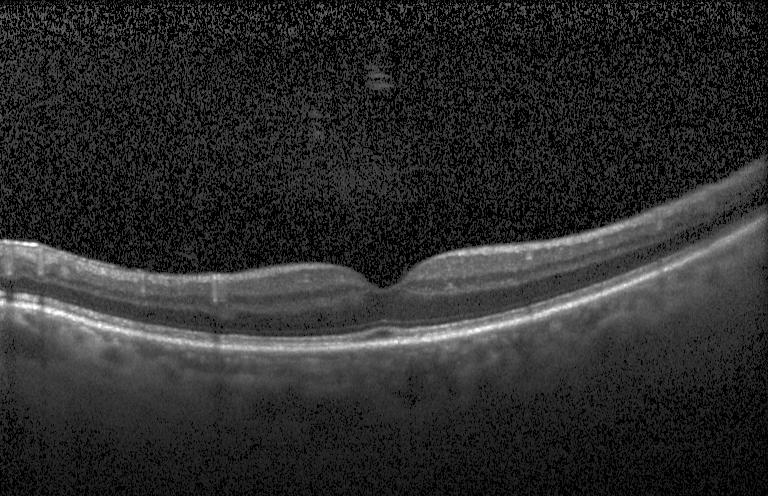 Diagnosis: no CNV, DME, or drusen.